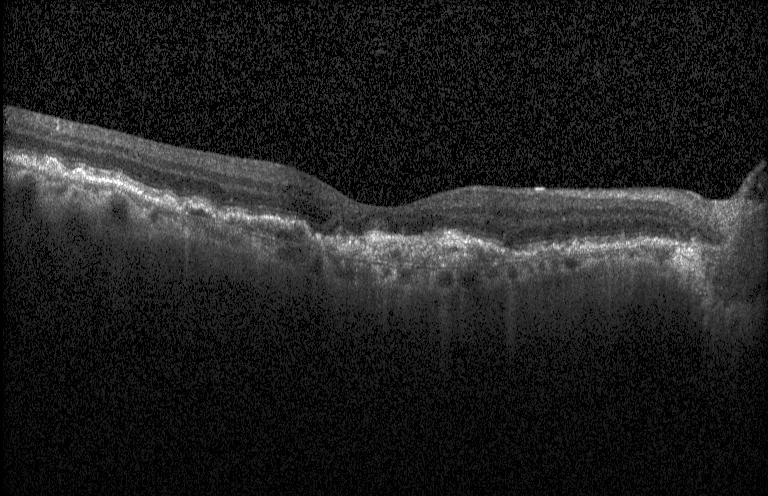
Retinal OCT cross-section. Heidelberg Spectralis OCT system. SD-OCT.
Diagnosis: a choroidal neovascular membrane.